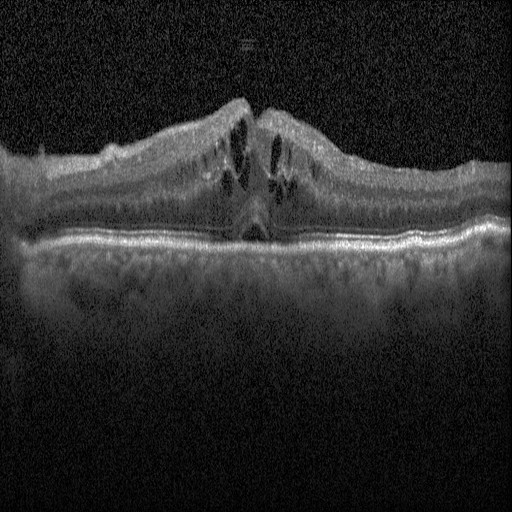
Optical coherence tomography scan.
This B-scan demonstrates DME.